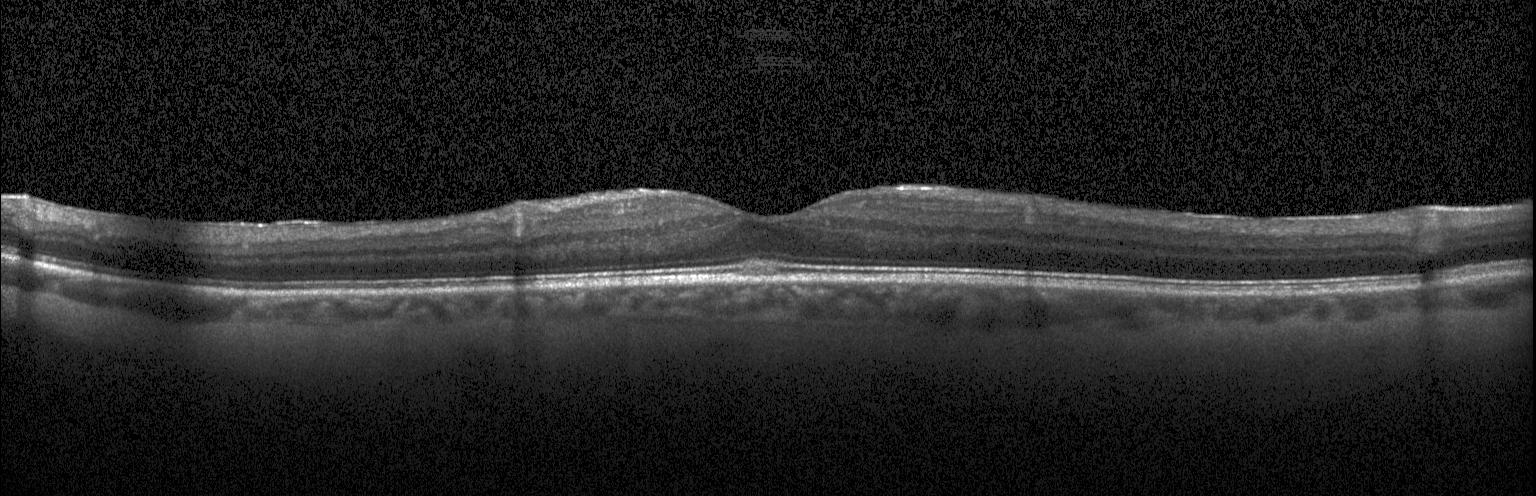

Finding: neither CNV, DME, nor drusen.